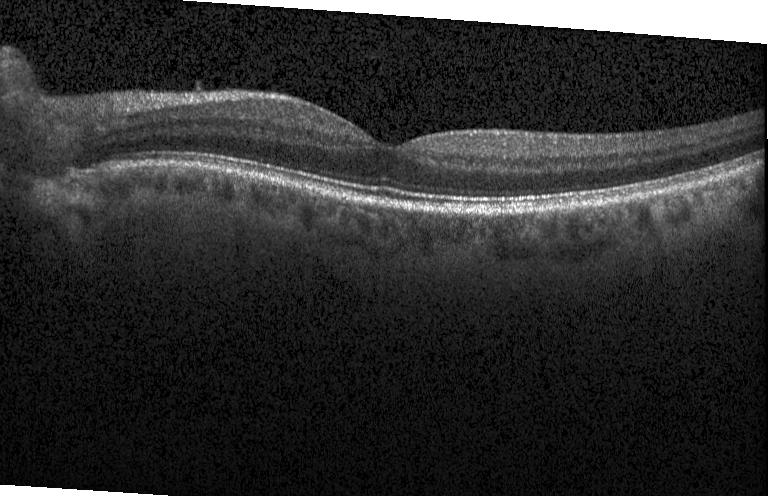 Through the macula. OCT B-scan. Spectral-domain OCT. Impression: no evidence of choroidal neovascularization, diabetic macular edema, or drusen.